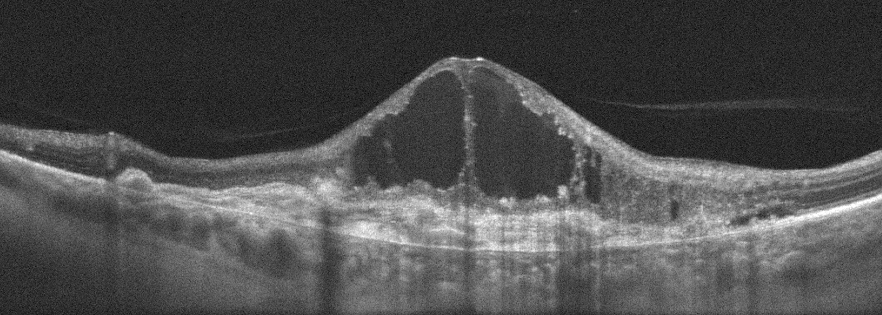 Retinal OCT cross-section, oculus sinister.
Impression: AMD.